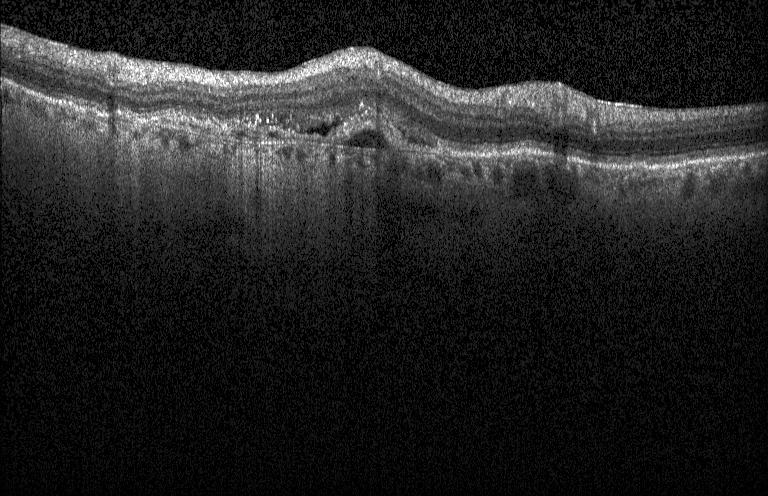
Optical coherence tomography B-scan — The scan shows CNV.